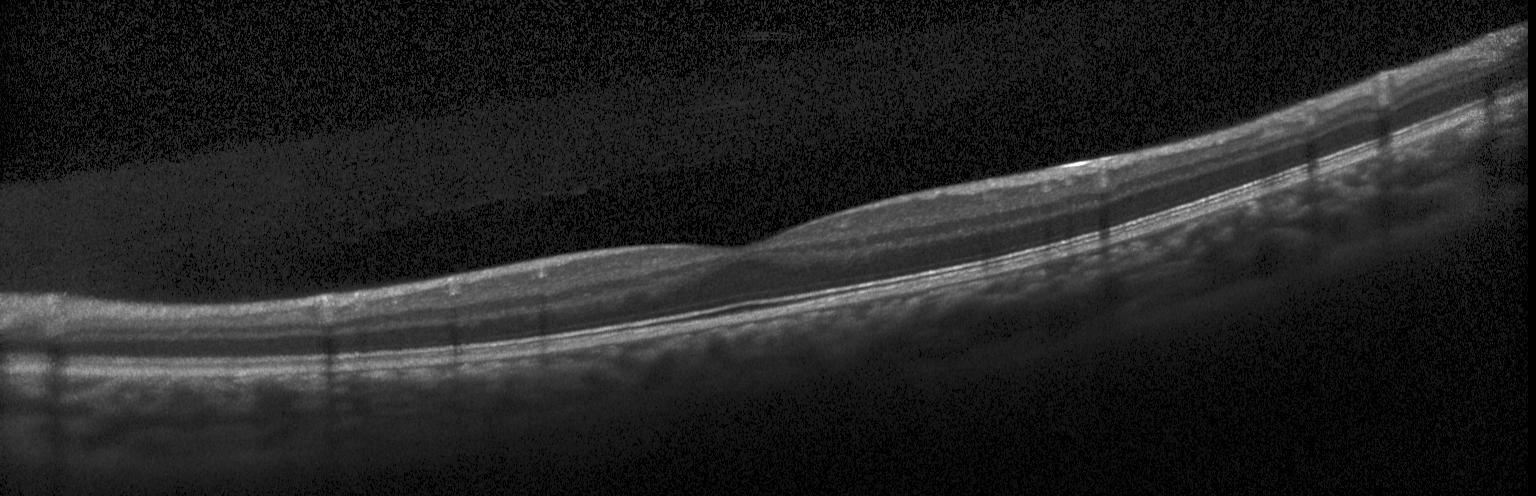 Acquired on a Heidelberg Spectralis; fovea-centered; retinal OCT cross-section. Assessment: no evidence of CNV, DME, or drusen.